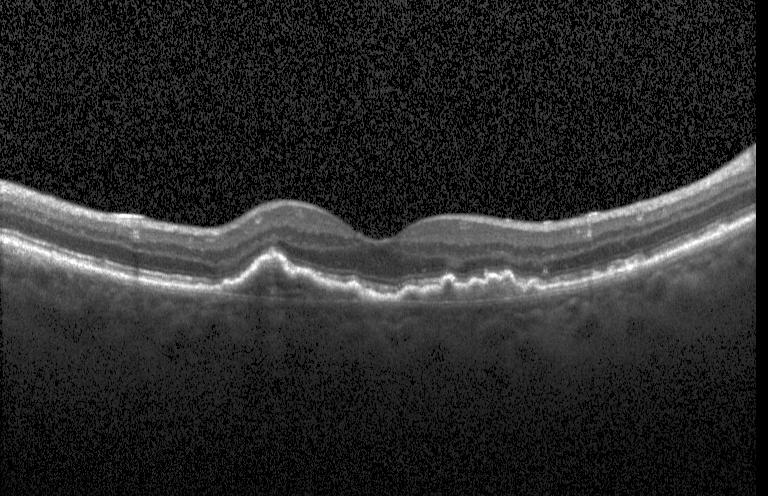

Macular OCT demonstrating a choroidal neovascular membrane.